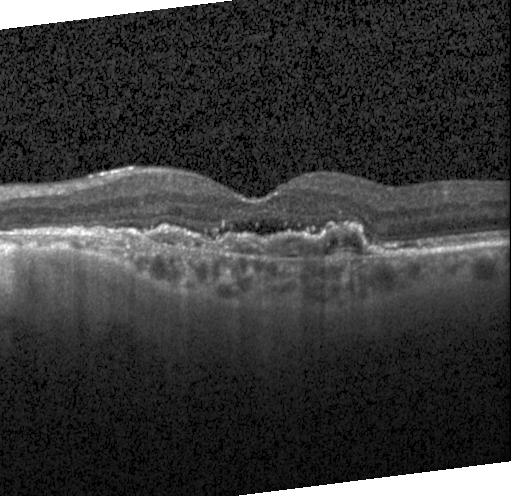 Spectral-domain OCT B-scan: a choroidal neovascular membrane.